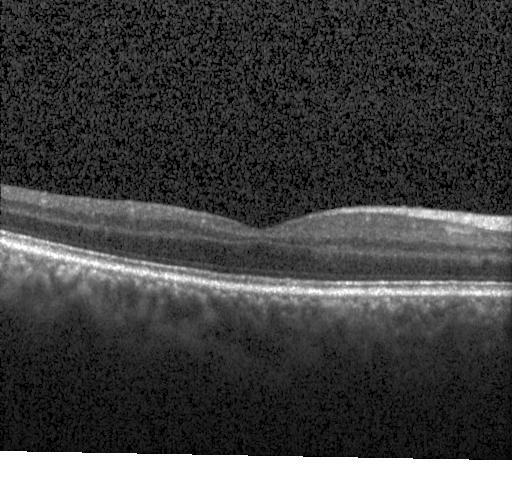
Optical coherence tomography B-scan. Spectral-domain OCT
Diagnosis: no choroidal neovascularization, no diabetic macular edema, and no drusen.